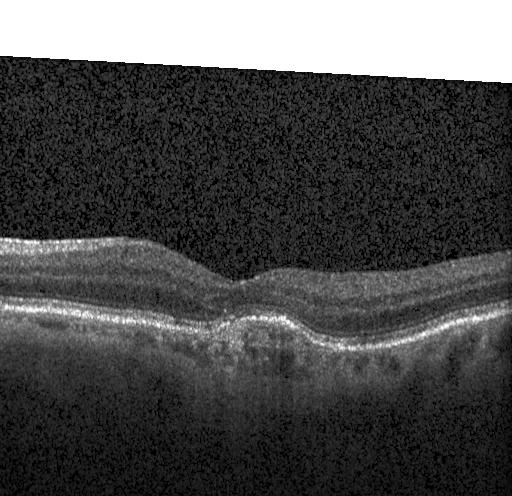

OCT finding: CNV.